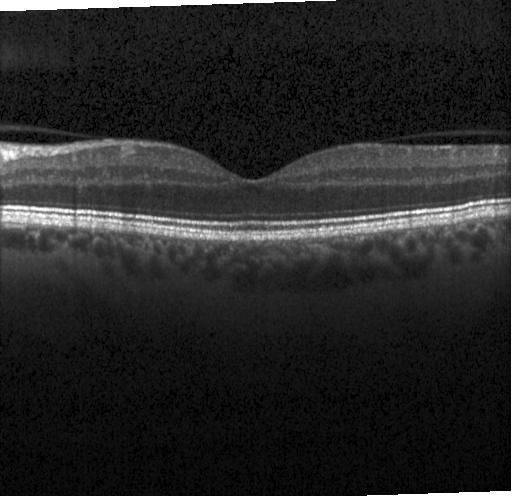 OCT finding: neither choroidal neovascularization, diabetic macular edema, nor drusen.